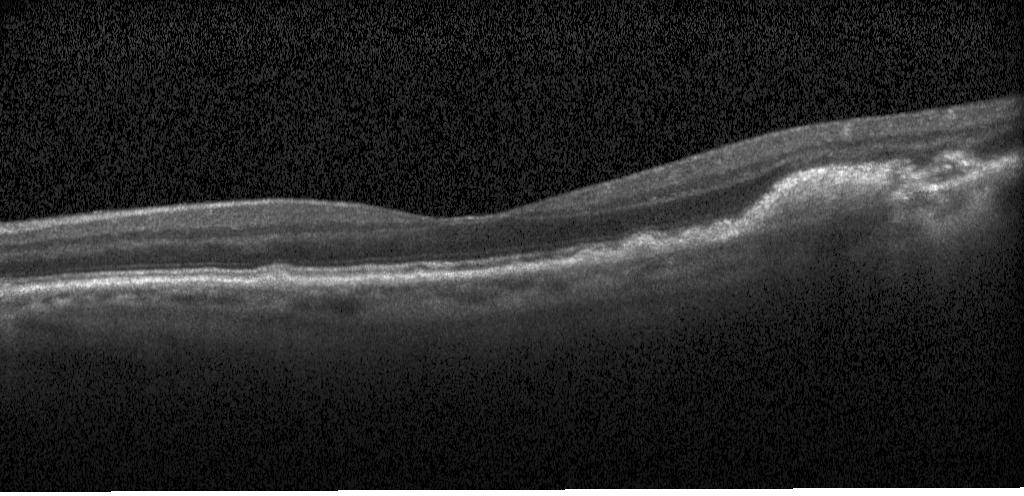 Macular OCT demonstrating CNV.